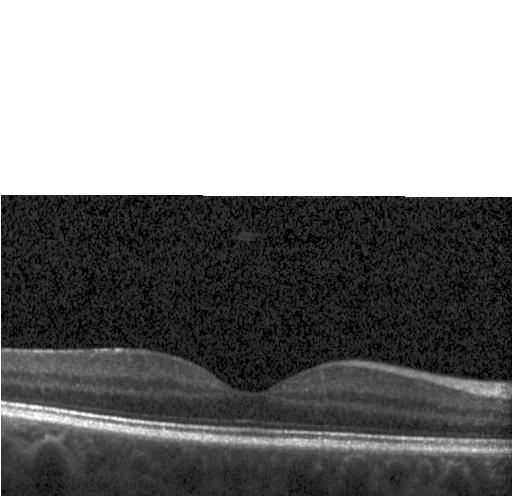 Optical coherence tomography scan
Dx: neither CNV, DME, nor drusen.